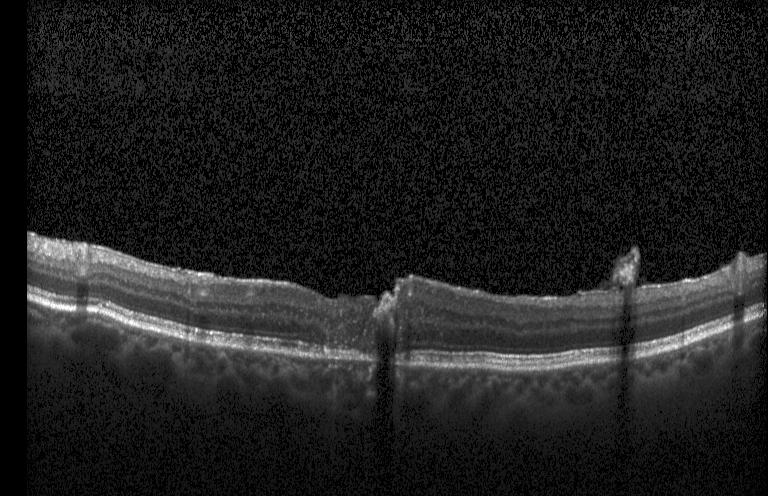
Horizontal scan through the fovea. Heidelberg Spectralis. Spectral-domain optical coherence tomography. Retinal OCT B-scan — Impression: choroidal neovascularization (CNV).